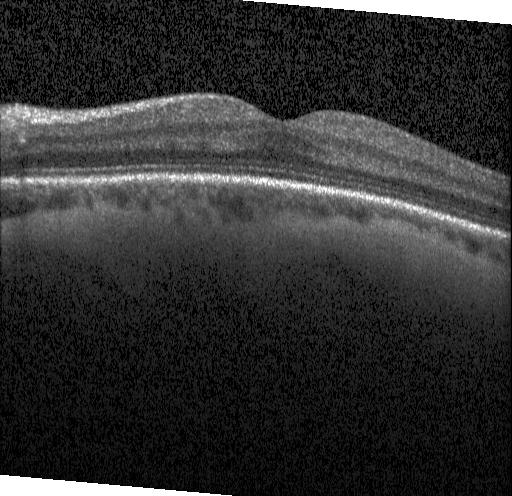

Finding: no CNV, no DME, and no drusen.